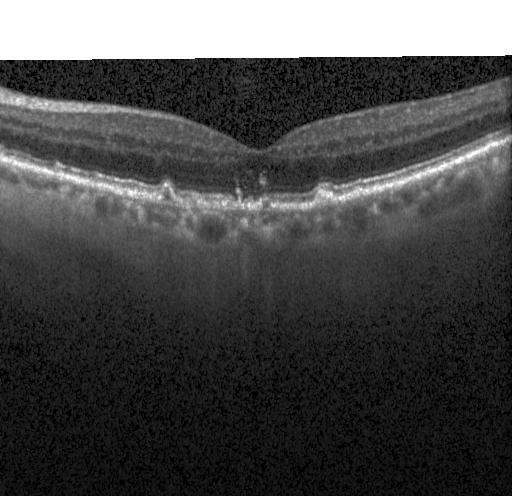 Spectral-domain OCT B-scan: drusen.